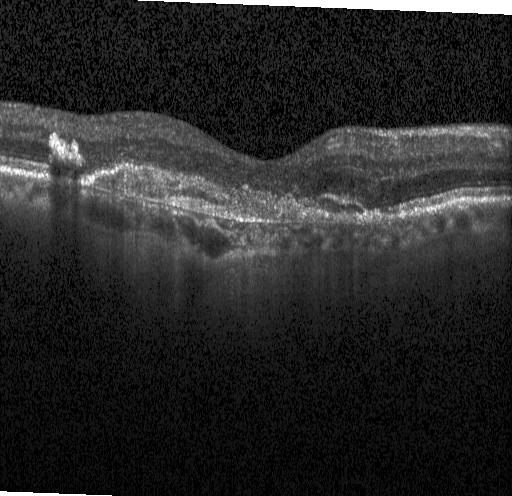 Impression: a choroidal neovascular membrane.